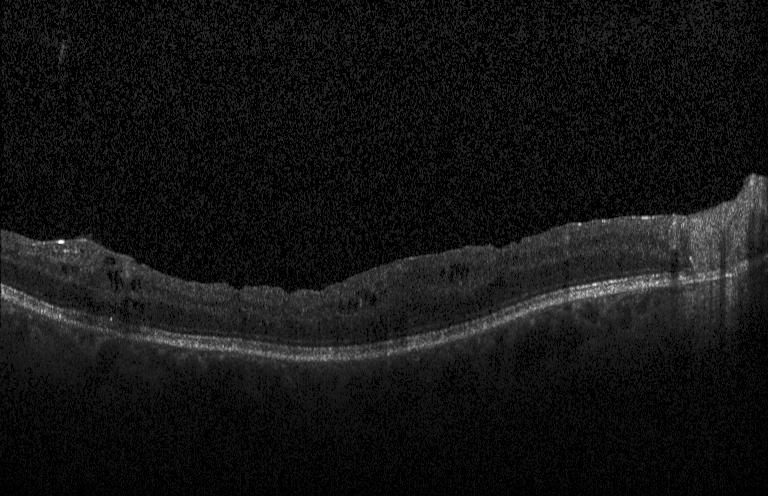

OCT finding: DME.